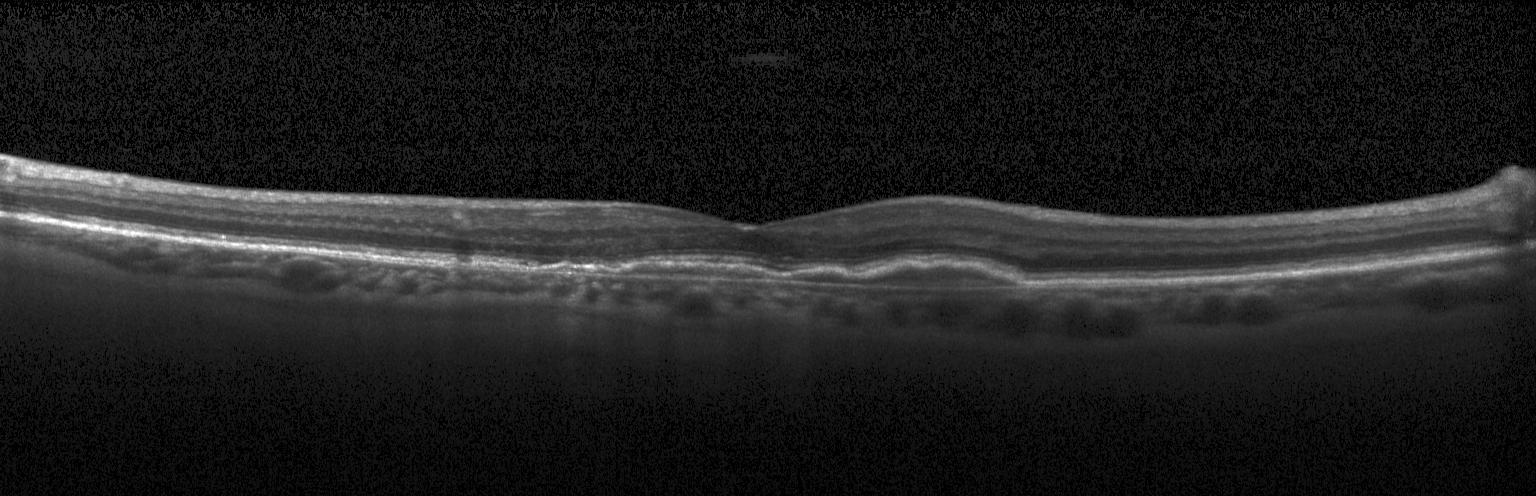 Spectral-domain OCT. Optical coherence tomography scan. Macular scan. A choroidal neovascular membrane.